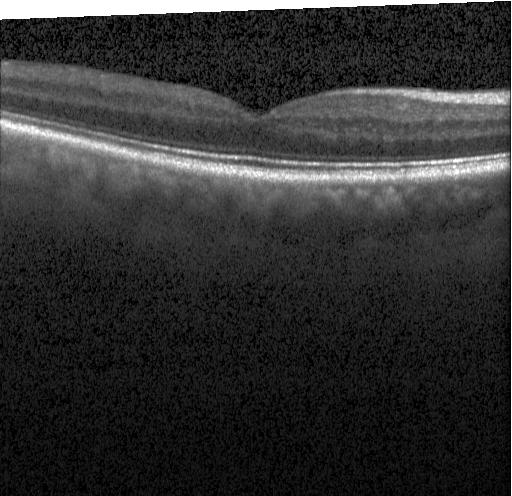
Diagnosis: neither choroidal neovascularization, diabetic macular edema, nor drusen.